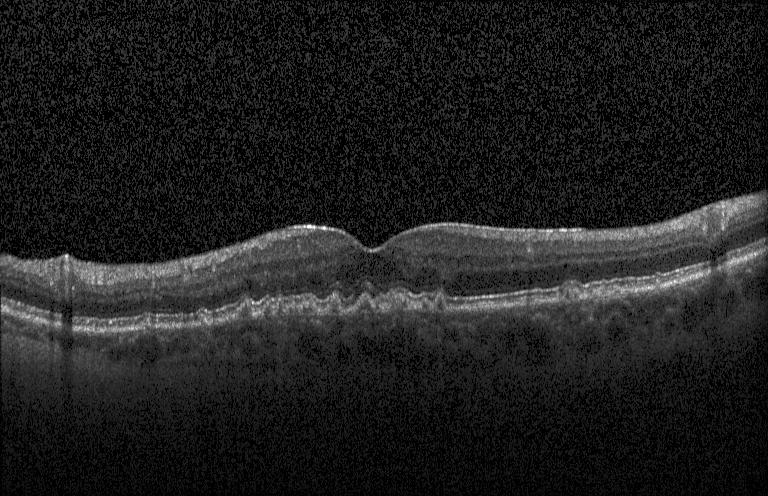

Macular OCT: drusen.